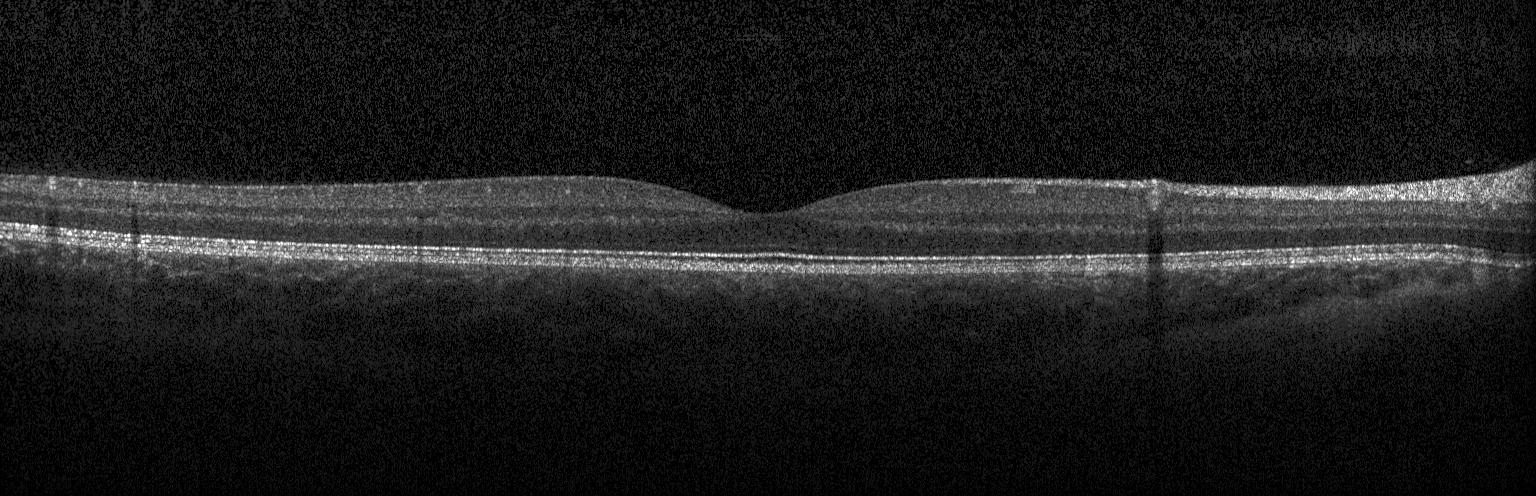
The scan shows no evidence of choroidal neovascularization, diabetic macular edema, or drusen.